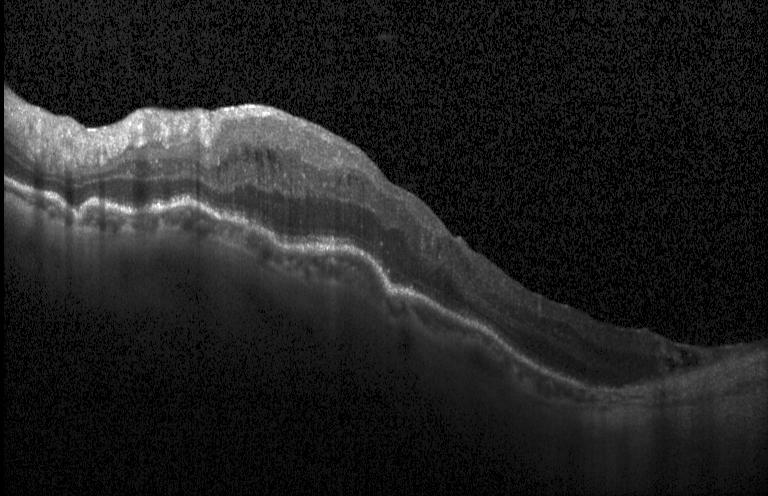 Heidelberg Spectralis; retinal OCT B-scan; spectral-domain optical coherence tomography; horizontal scan through the fovea. Diagnosis: a choroidal neovascular membrane.